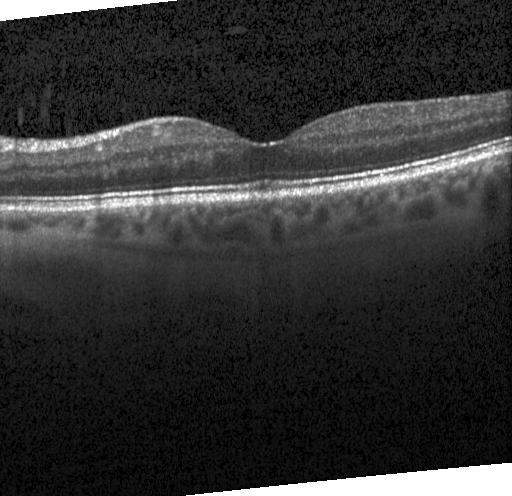

Macular OCT: no choroidal neovascularization, no diabetic macular edema, and no drusen.